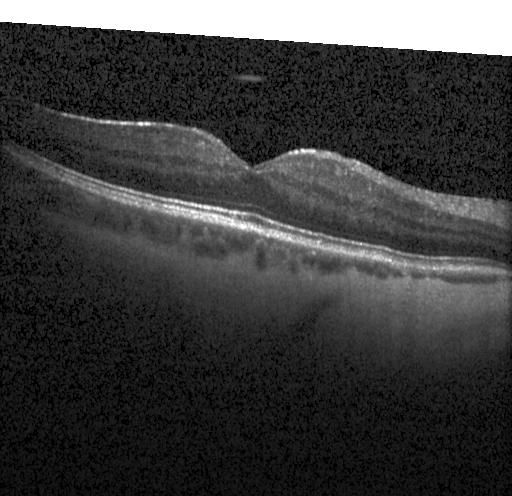

Diagnosis: no evidence of choroidal neovascularization, diabetic macular edema, or drusen.